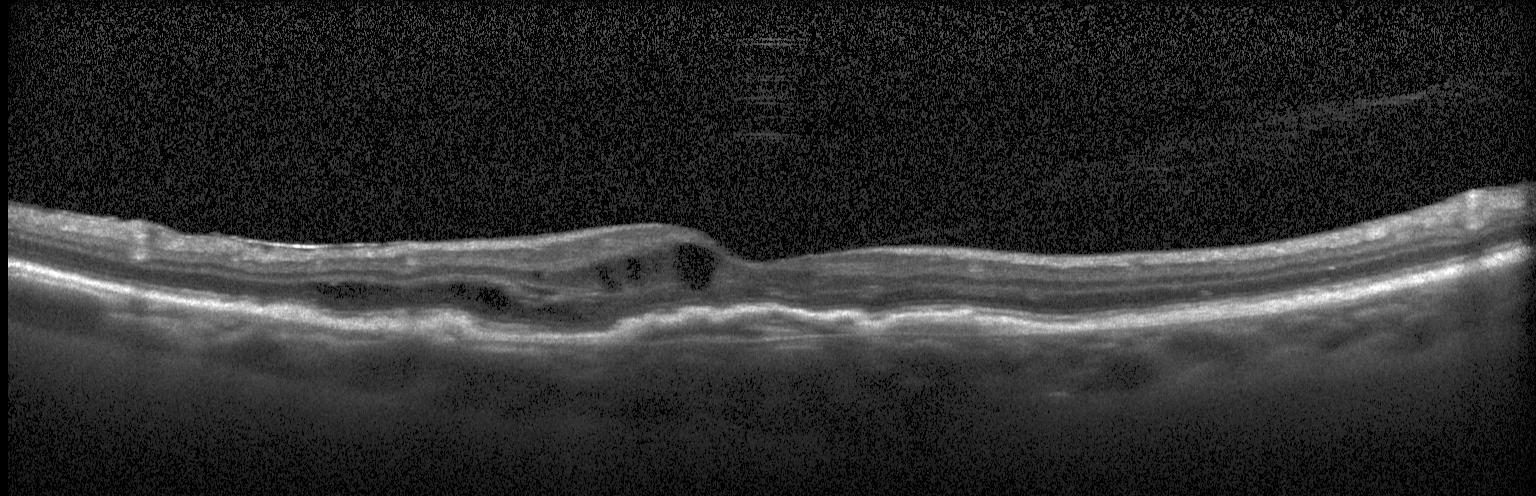

Assessment: CNV.